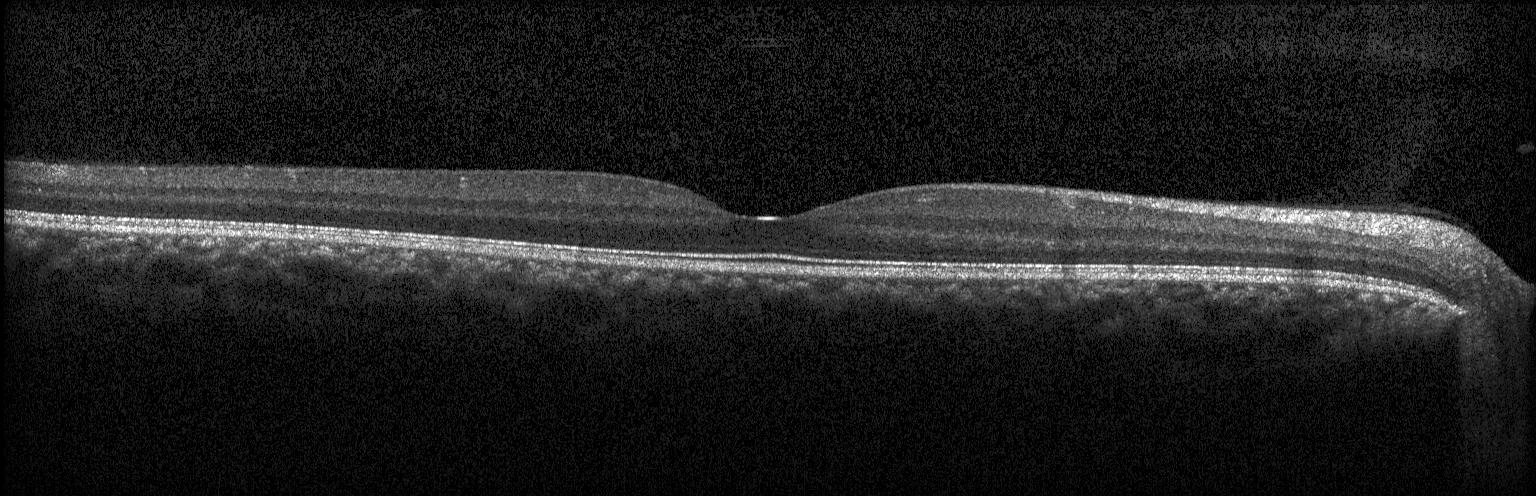 Optical coherence tomography B-scan · fovea-centered · Heidelberg Spectralis OCT system · SD-OCT.
Diagnosis: no CNV, DME, or drusen.